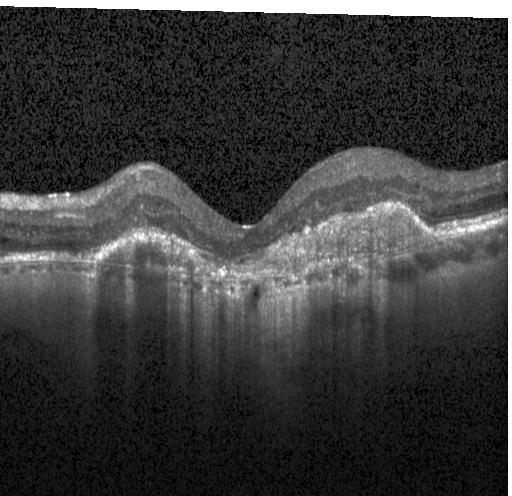
Finding: choroidal neovascularization.